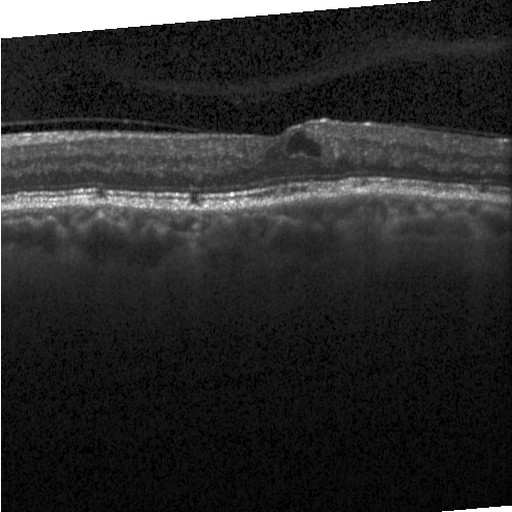
Diabetic macular edema (DME).